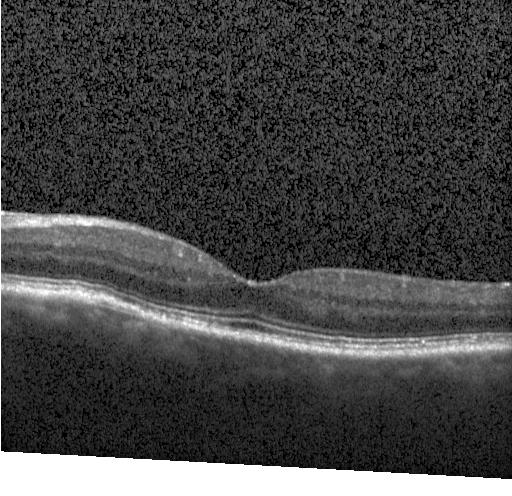 Optical coherence tomography scan · spectral-domain optical coherence tomography — Assessment: multiple drusen.